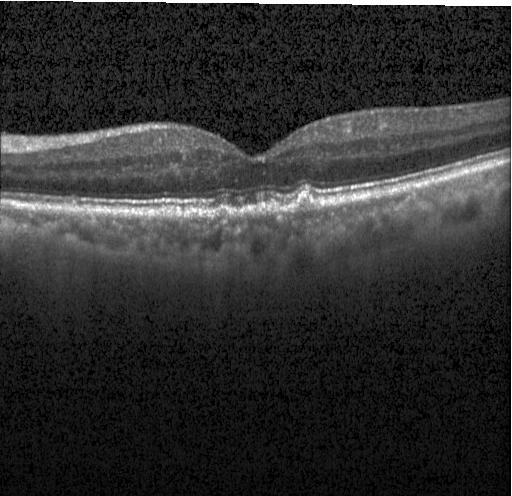 Optical coherence tomography B-scan. Macular scan
Macular OCT: drusen.